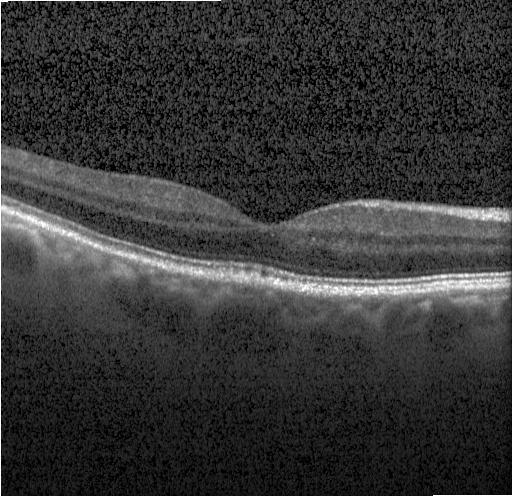 OCT line scan. Finding: no CNV, no DME, and no drusen.